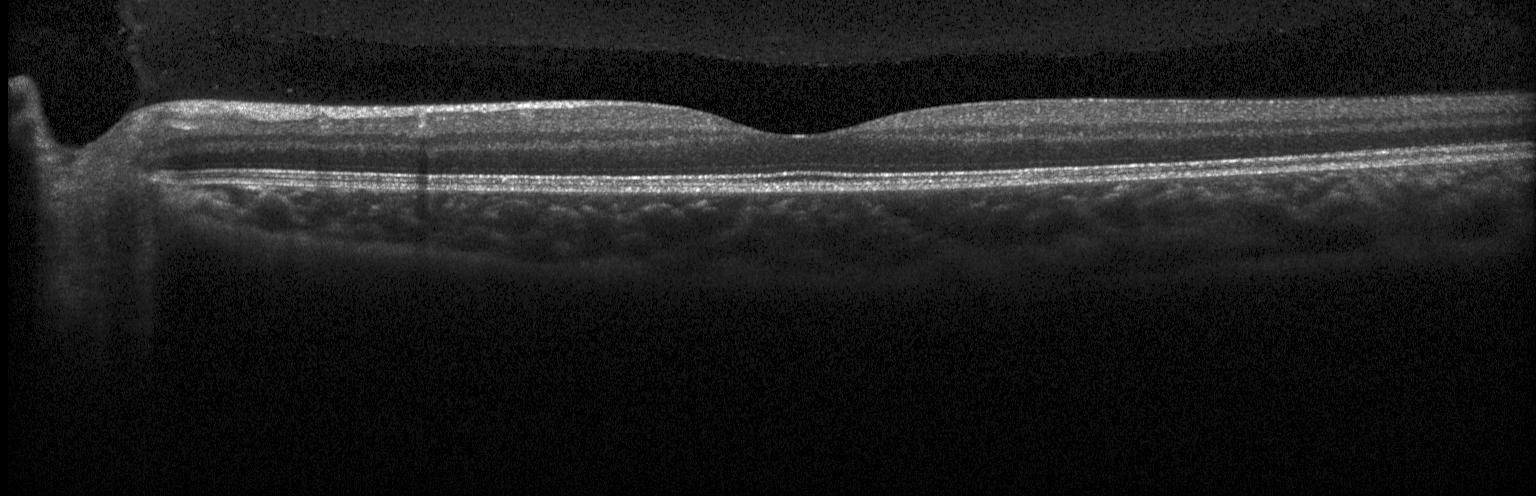 Heidelberg Spectralis, centered on the fovea, retinal OCT cross-section.
Macular OCT: no choroidal neovascularization, no diabetic macular edema, and no drusen.